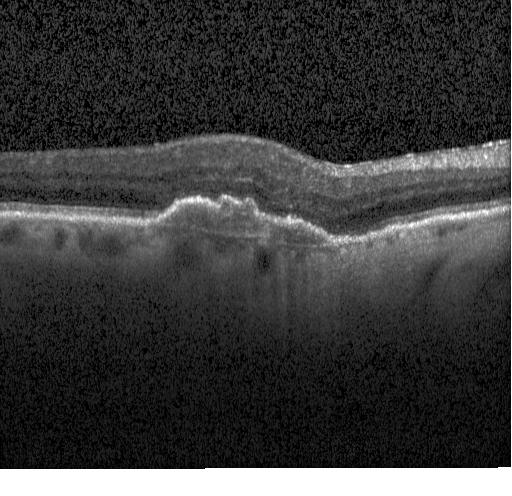 Spectral-domain OCT B-scan: choroidal neovascularization.